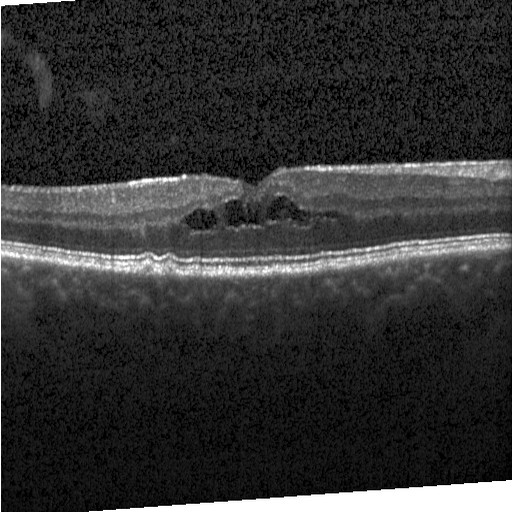

Macular scan. Spectral-domain optical coherence tomography. Optical coherence tomography scan. The scan shows diabetic macular edema (DME).